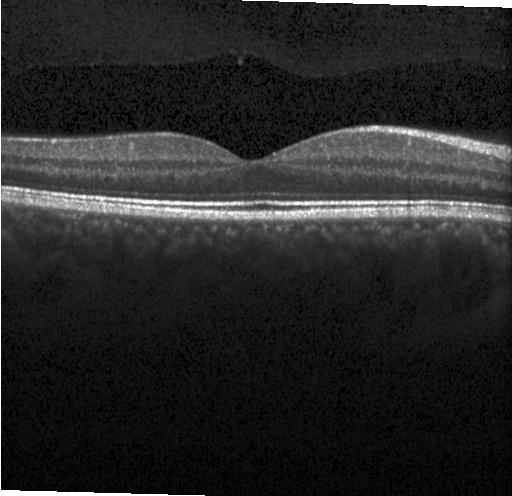
This B-scan demonstrates no CNV, DME, or drusen.